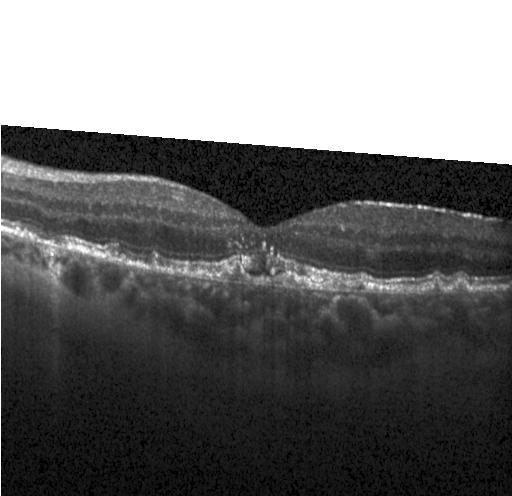
Spectral-domain OCT. Acquired on a Heidelberg Spectralis. Retinal OCT cross-section. Finding: a choroidal neovascular membrane.